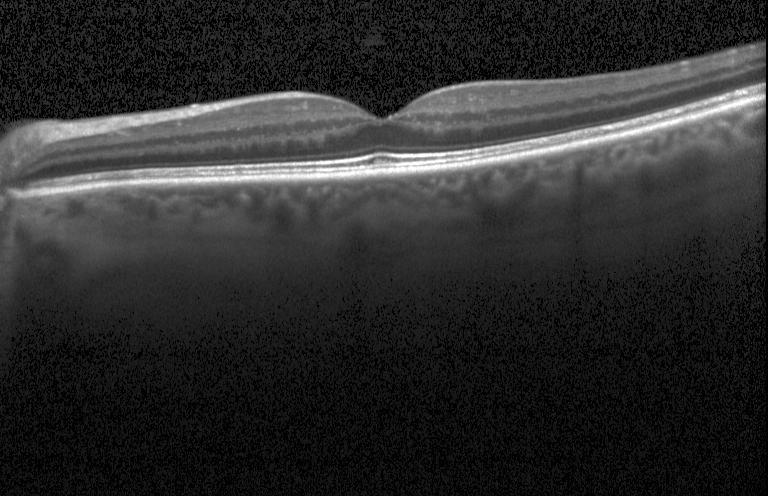

OCT B-scan showing neither CNV, DME, nor drusen.